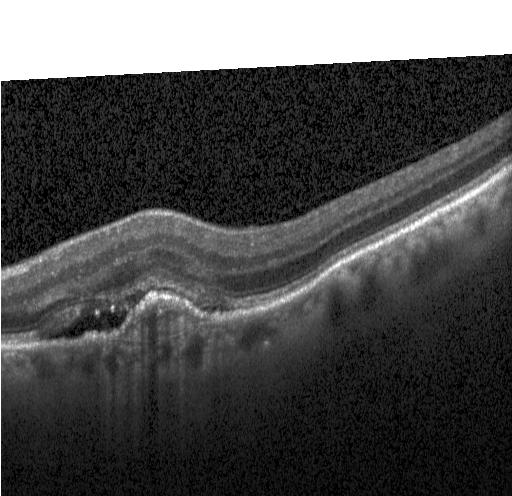
Spectral-domain OCT. Retinal OCT cross-section.
A choroidal neovascular membrane.